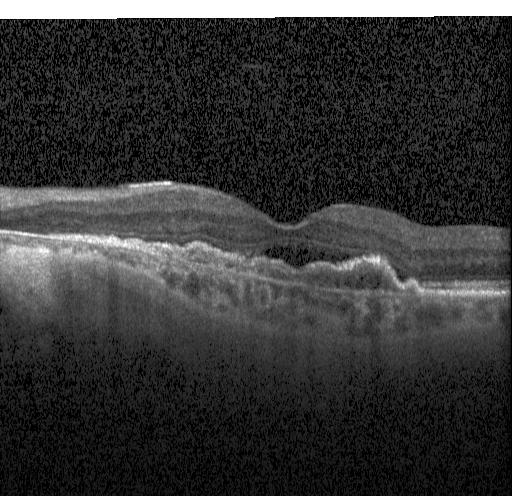 Diagnosis: a choroidal neovascular membrane.